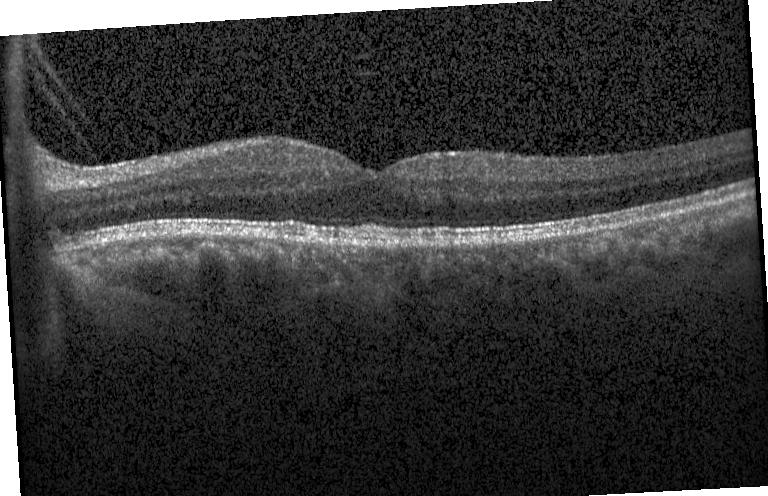
Optical coherence tomography B-scan. Macular scan. Instrument: Heidelberg Spectralis. SD-OCT — This B-scan demonstrates neither choroidal neovascularization, diabetic macular edema, nor drusen.